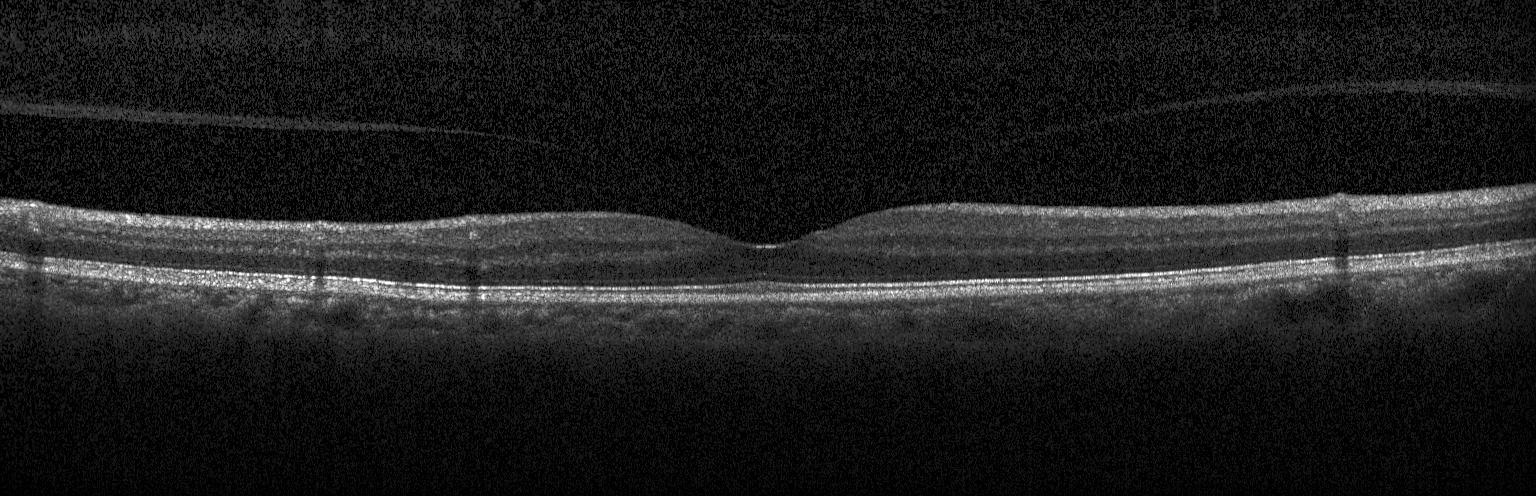 Retinal OCT cross-section showing no evidence of choroidal neovascularization, diabetic macular edema, or drusen.